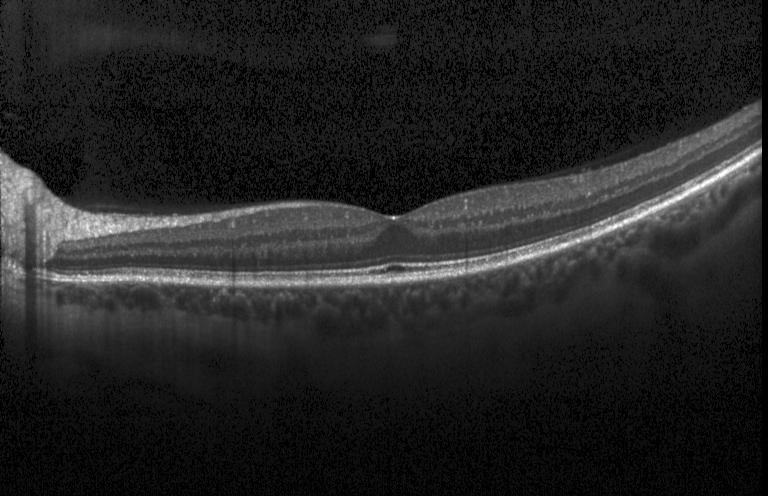
SD-OCT; retinal OCT B-scan. Dx: no choroidal neovascularization, no diabetic macular edema, and no drusen.